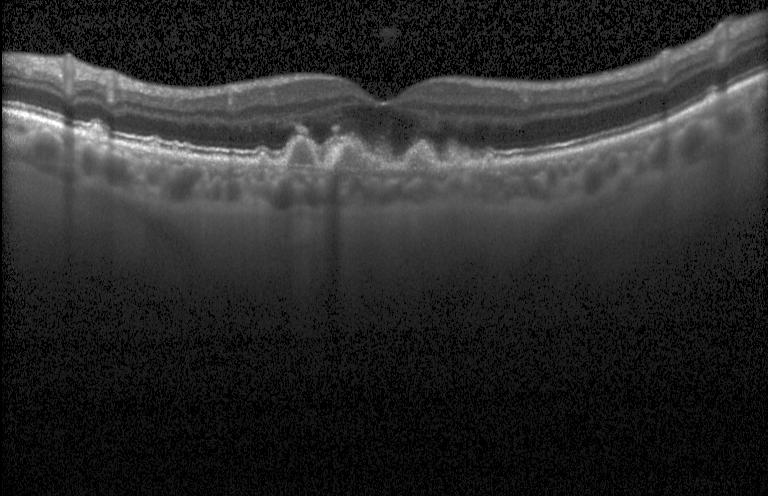 OCT B-scan. Diagnosis: multiple drusen.